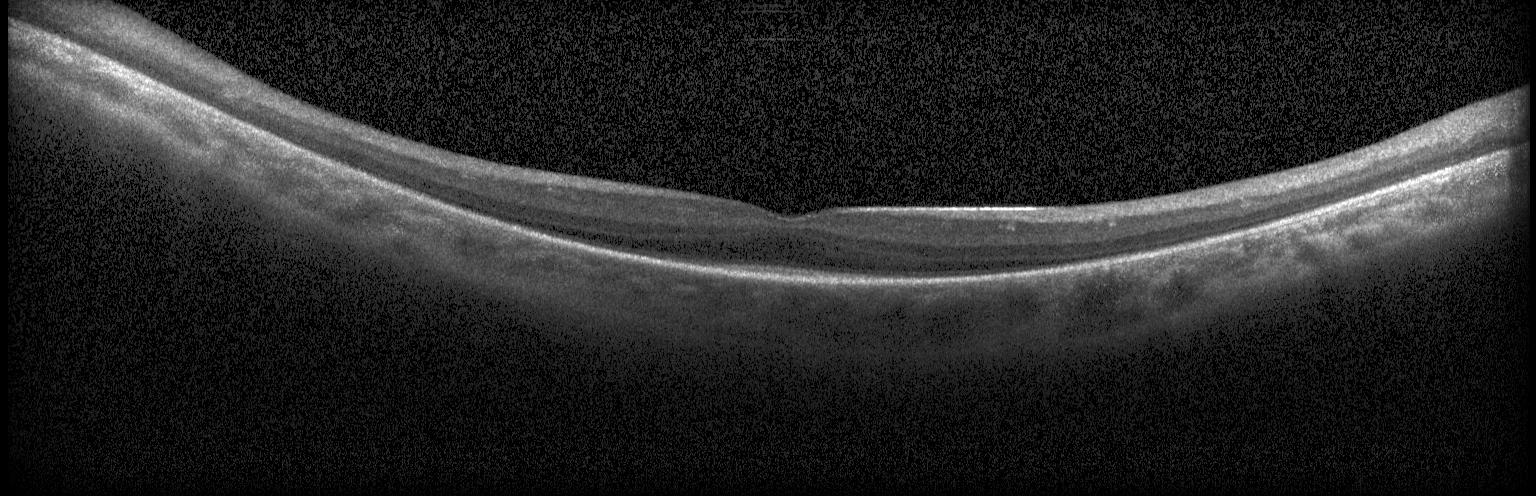 Retinal OCT cross-section · fovea-centered — Dx: no CNV, no DME, and no drusen.